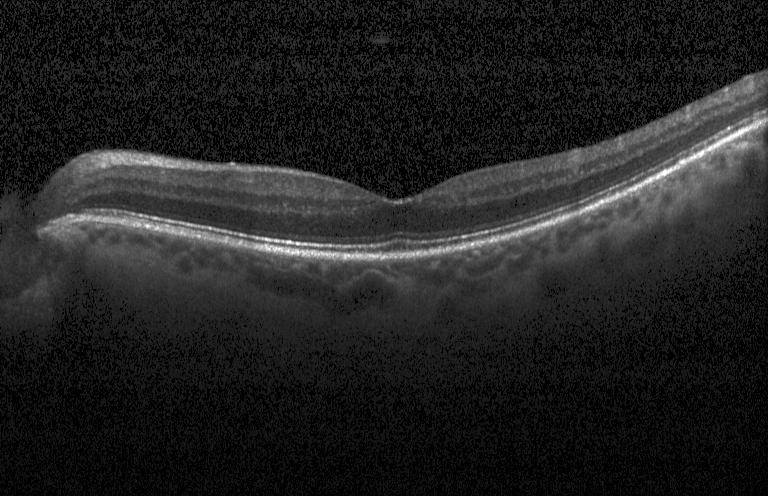

Macular scan; retinal OCT cross-section. Diagnosis: neither choroidal neovascularization, diabetic macular edema, nor drusen.